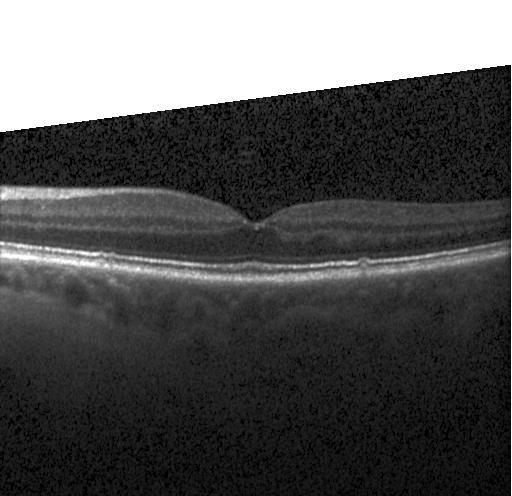 Retinal OCT B-scan — Dx: drusen.